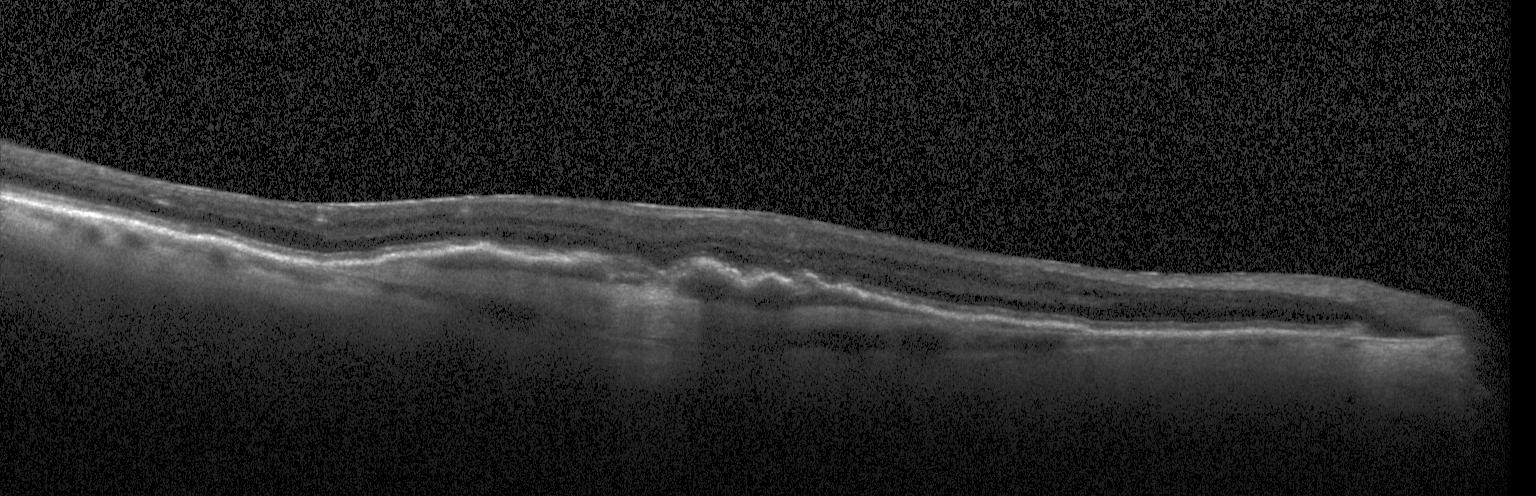
Dx: a choroidal neovascular membrane.